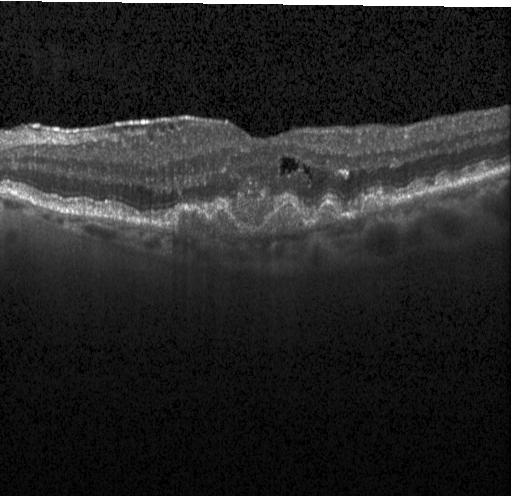 Assessment: a choroidal neovascular membrane.